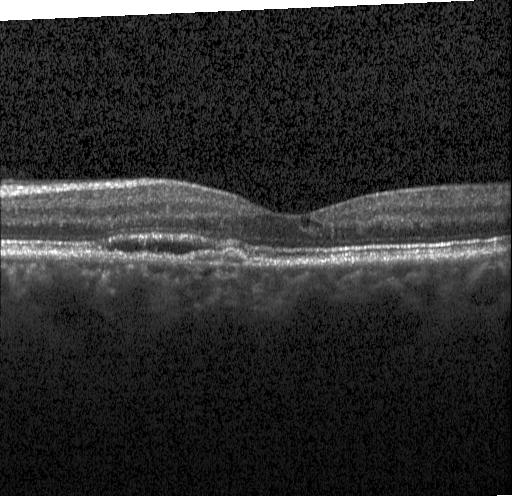

Diagnosis: a choroidal neovascular membrane.